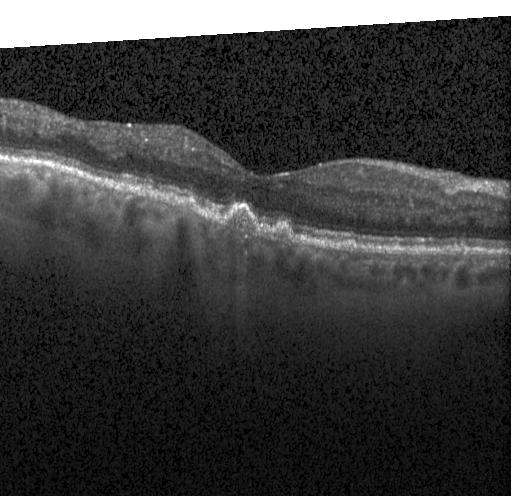

Diagnosis: sub-RPE drusenoid deposits.